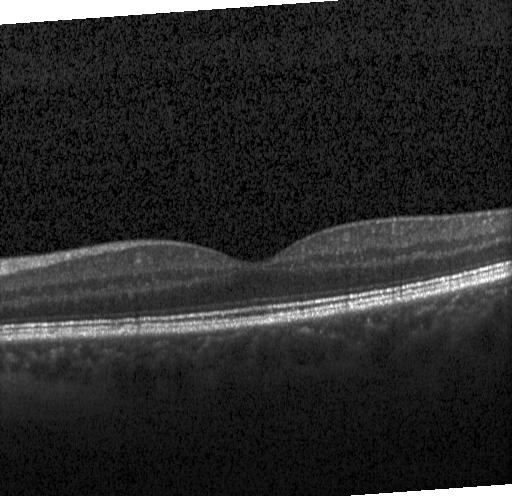

Retinal OCT B-scan — Finding: no choroidal neovascularization, no diabetic macular edema, and no drusen.